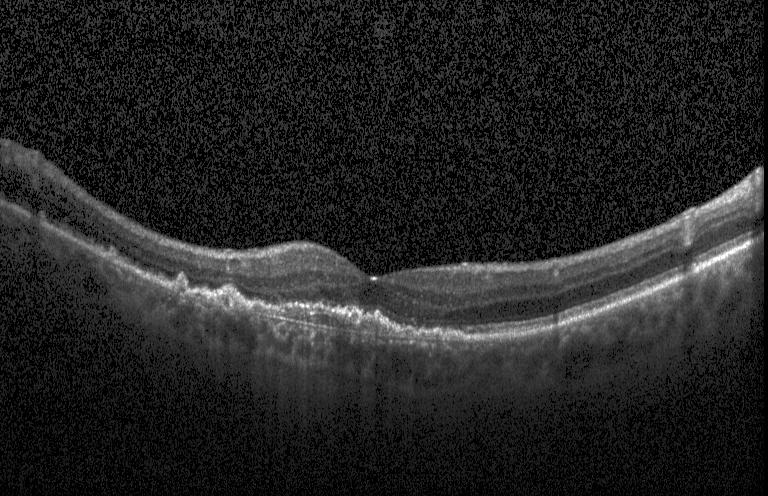 Impression: a choroidal neovascular membrane.